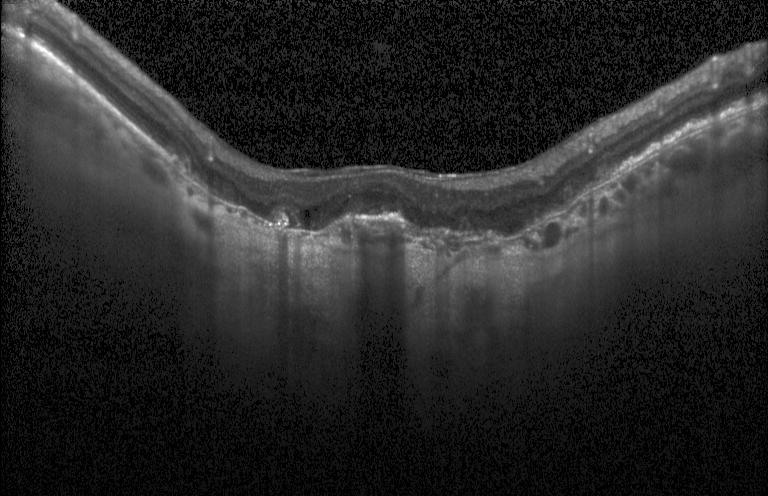 Retinal OCT cross-section showing choroidal neovascularization (CNV).